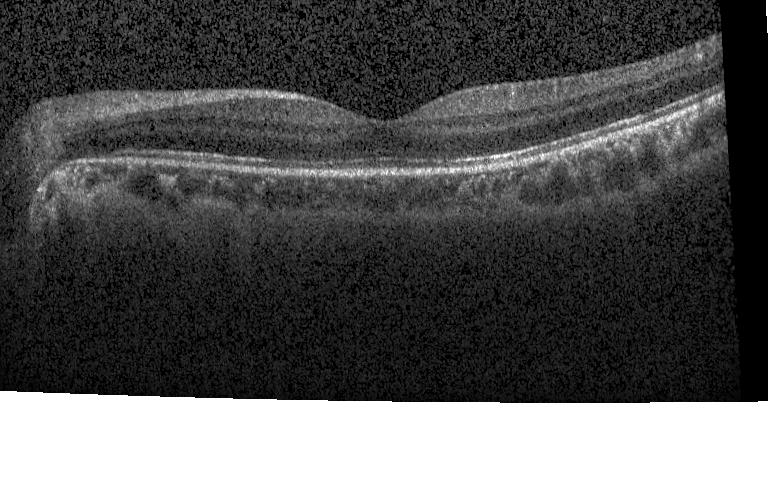 Spectral-domain OCT; macular scan; OCT B-scan.
OCT finding: no evidence of CNV, DME, or drusen.